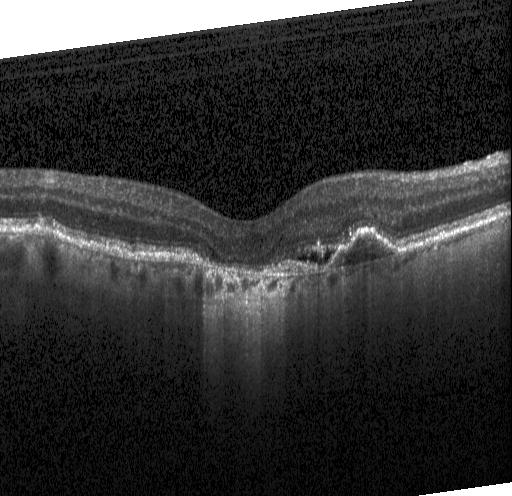 Heidelberg Spectralis OCT system, through the macula, optical coherence tomography scan — Assessment: a choroidal neovascular membrane.